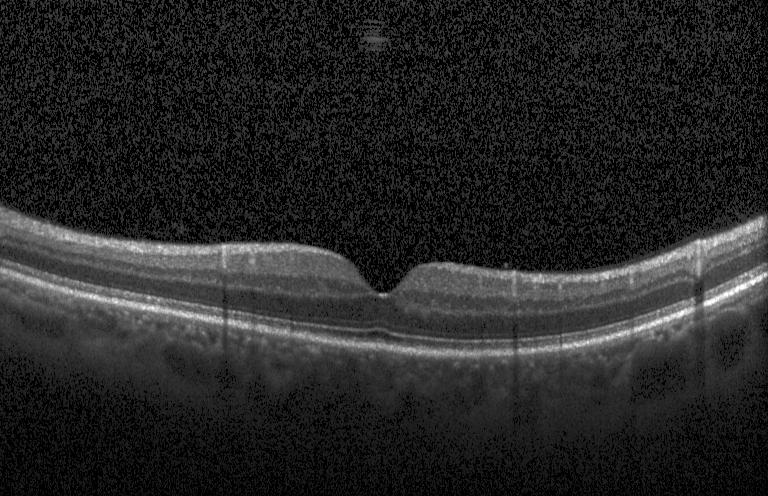

Impression: no evidence of choroidal neovascularization, diabetic macular edema, or drusen.